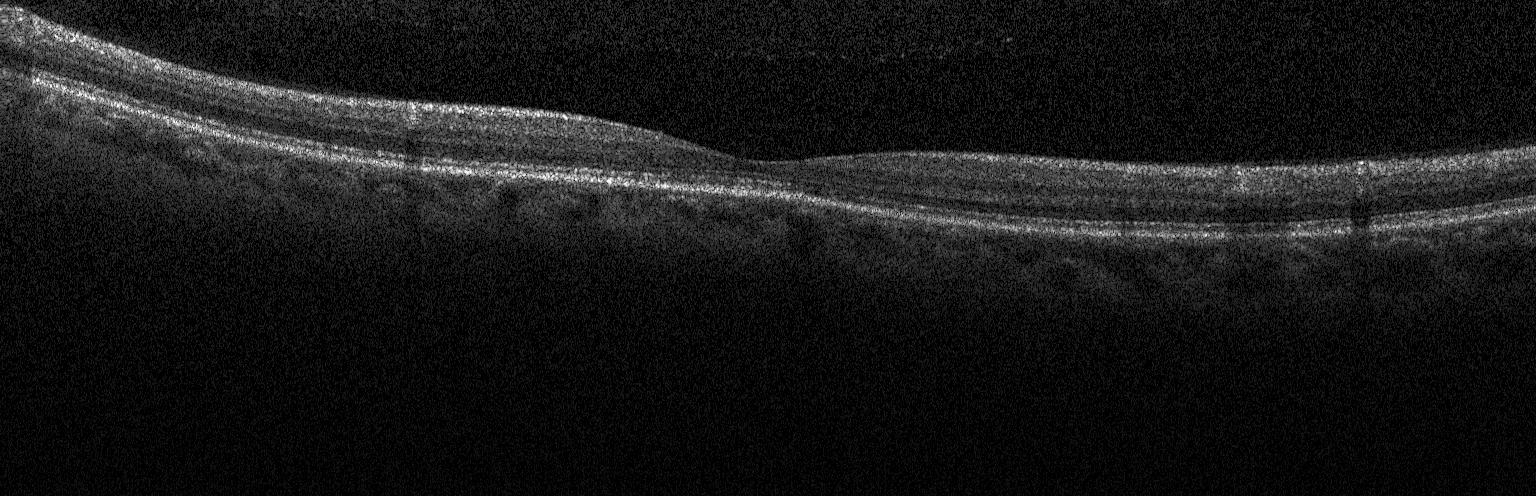
OCT line scan. Macular OCT: no evidence of CNV, DME, or drusen.